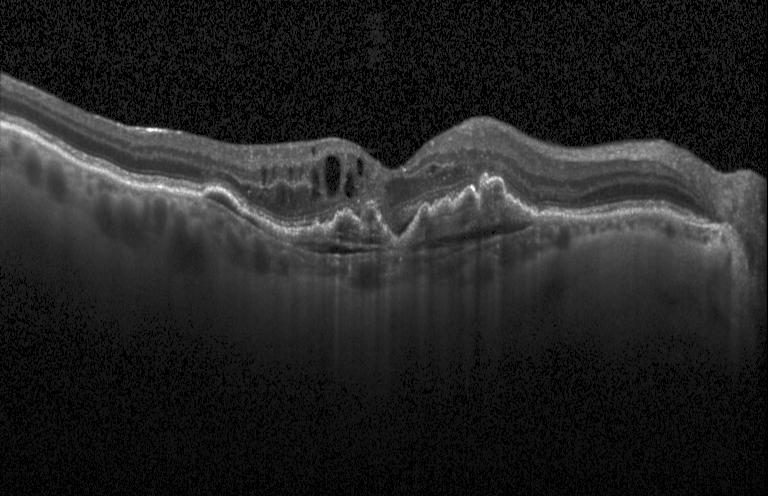

Impression: choroidal neovascularization (CNV).